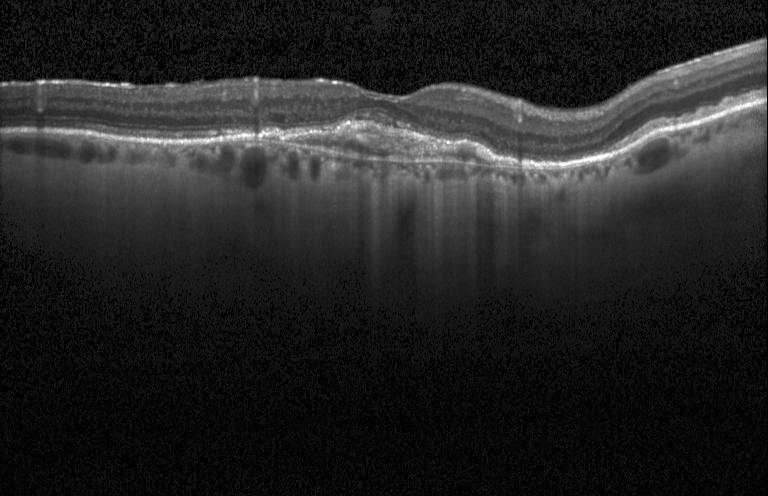
Optical coherence tomography B-scan — Diagnosis: a choroidal neovascular membrane.